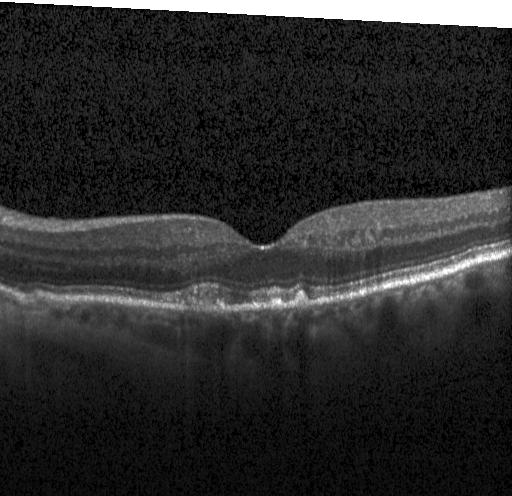

Centered on the fovea. Optical coherence tomography B-scan. SD-OCT. Heidelberg Spectralis.
Diagnosis: multiple drusen.